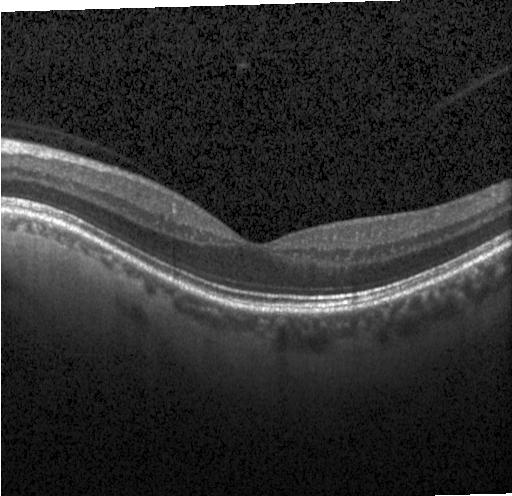

Retinal OCT B-scan; SD-OCT. Finding: no CNV, DME, or drusen.